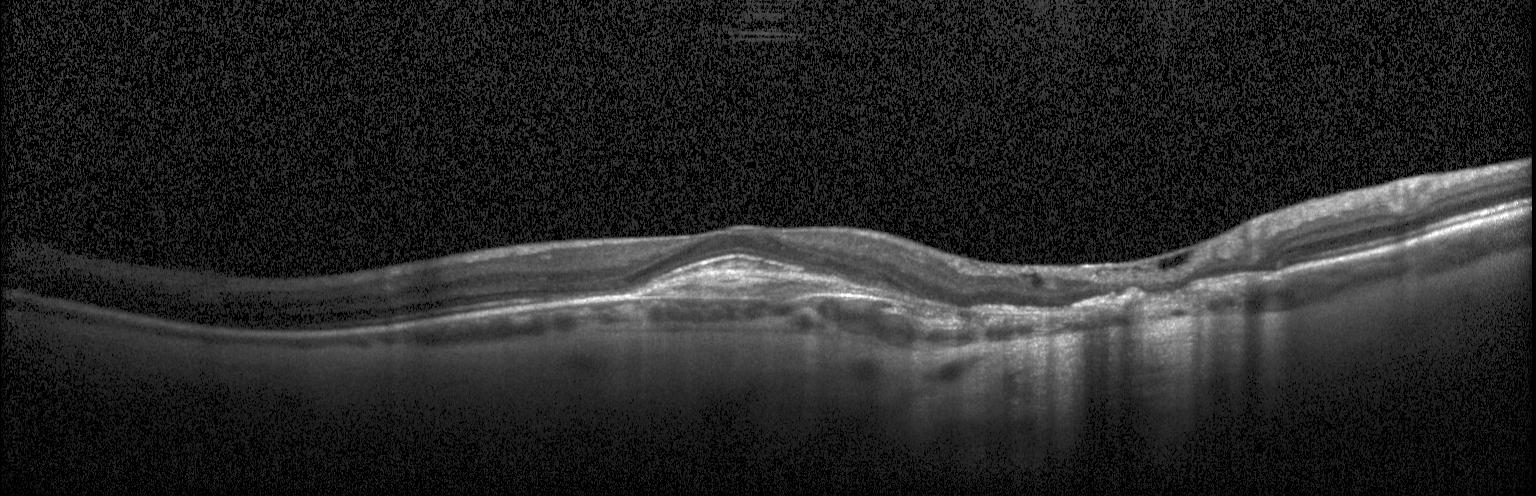

SD-OCT, acquired on a Heidelberg Spectralis, OCT B-scan. Assessment: a choroidal neovascular membrane.